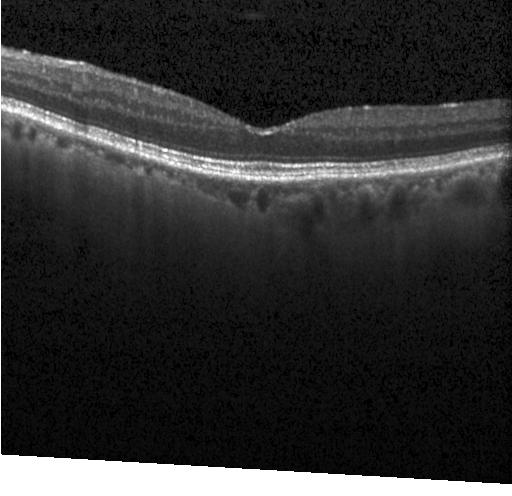 OCT B-scan showing neither CNV, DME, nor drusen.